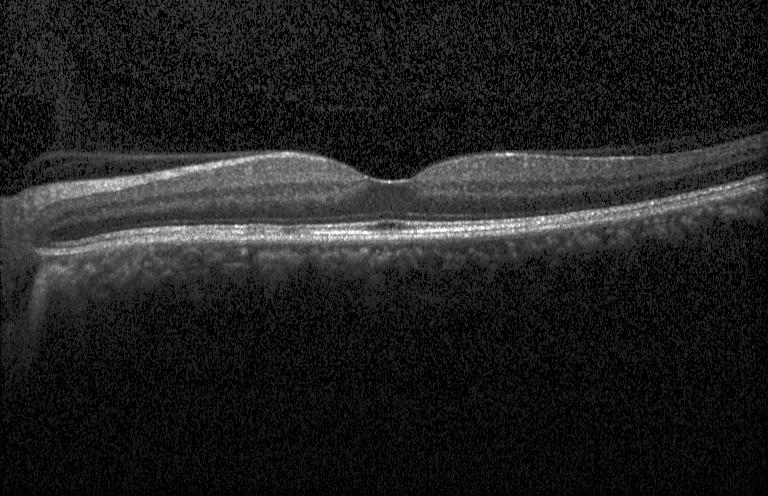
Spectral-domain optical coherence tomography. Acquired on a Heidelberg Spectralis. OCT line scan. Diagnosis: neither CNV, DME, nor drusen.